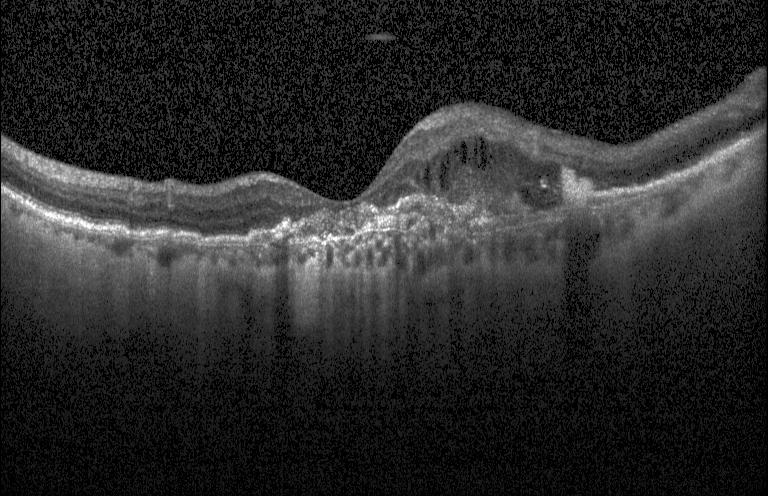
OCT B-scan; acquired on a Heidelberg Spectralis; fovea-centered. OCT finding: CNV.